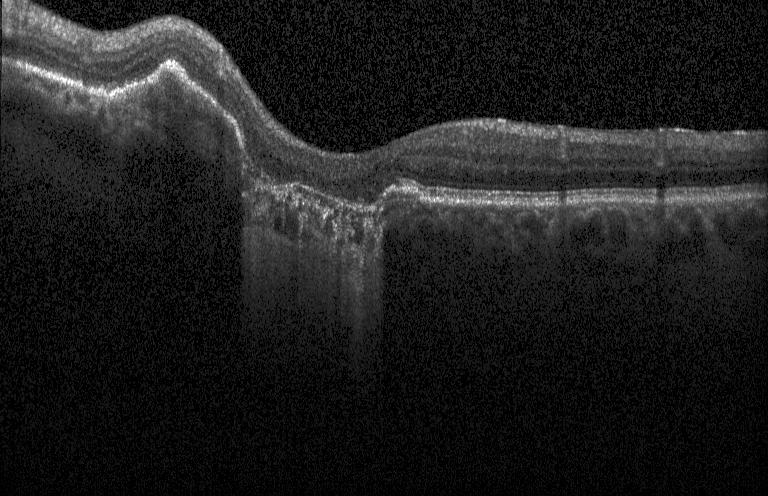 Retinal OCT B-scan · macular scan · Heidelberg Spectralis
The scan shows a choroidal neovascular membrane.